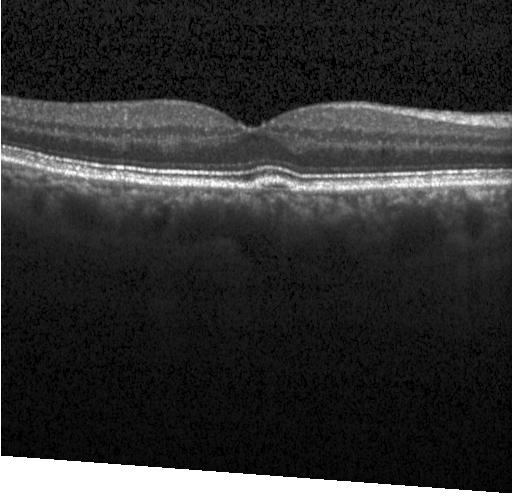

OCT line scan, acquired on a Heidelberg Spectralis, SD-OCT, fovea-centered. Macular OCT: no CNV, no DME, and no drusen.